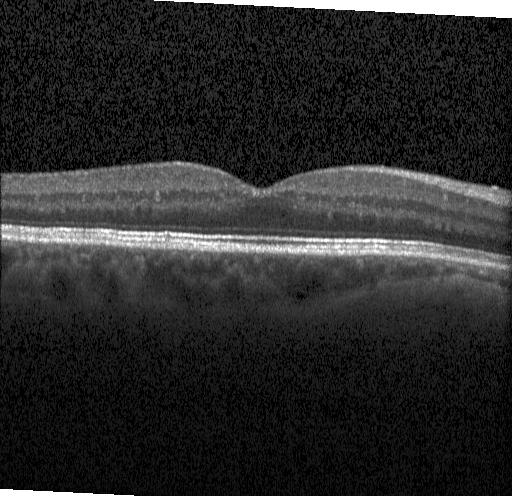

Spectral-domain OCT. OCT B-scan. Centered on the fovea
Diagnosis: no CNV, DME, or drusen.